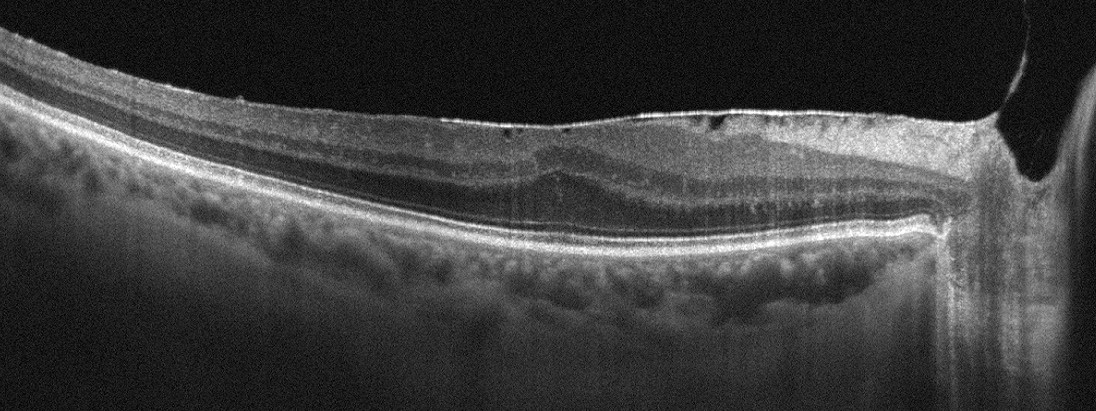 Impression: epiretinal membrane (ERM).